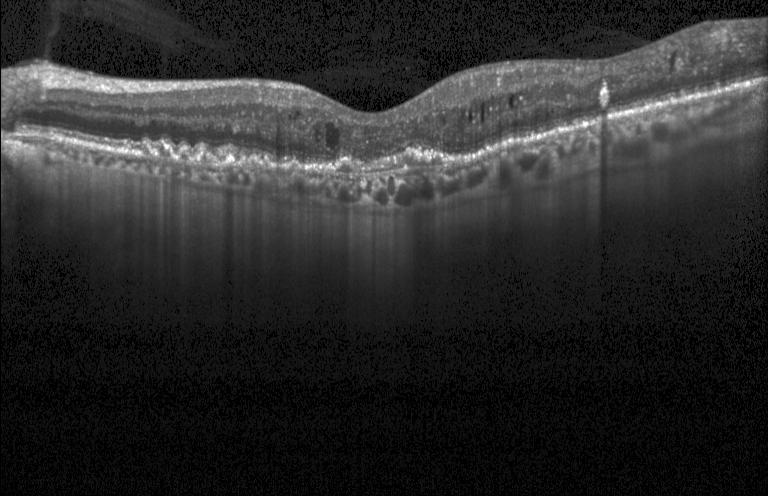

Macular OCT: a choroidal neovascular membrane.